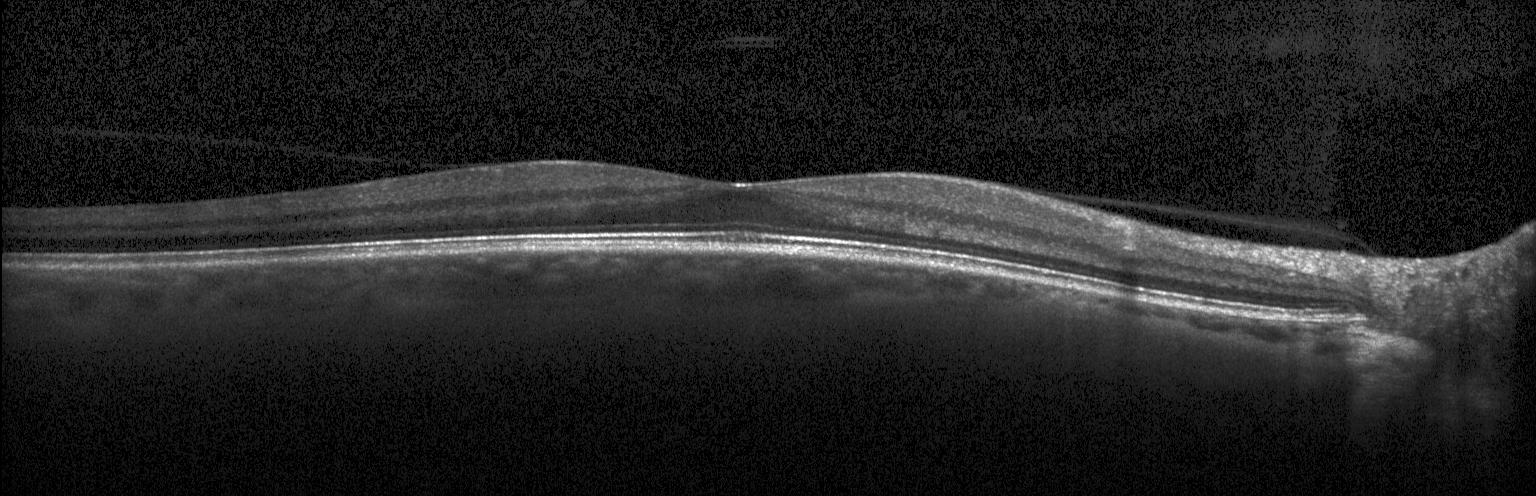 OCT finding: no CNV, no DME, and no drusen.